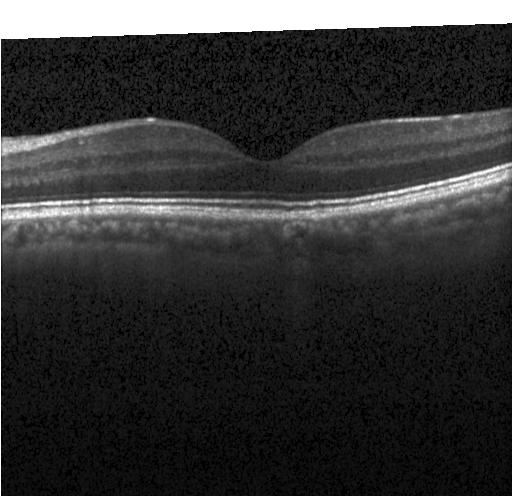 Finding: no evidence of CNV, DME, or drusen.